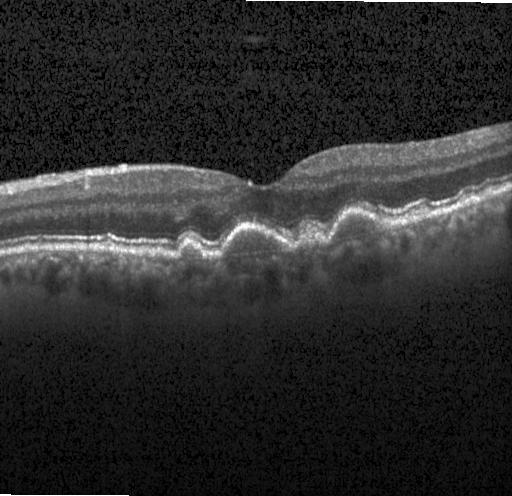 Heidelberg Spectralis OCT system, macular scan, spectral-domain optical coherence tomography, optical coherence tomography B-scan
Impression: multiple drusen.